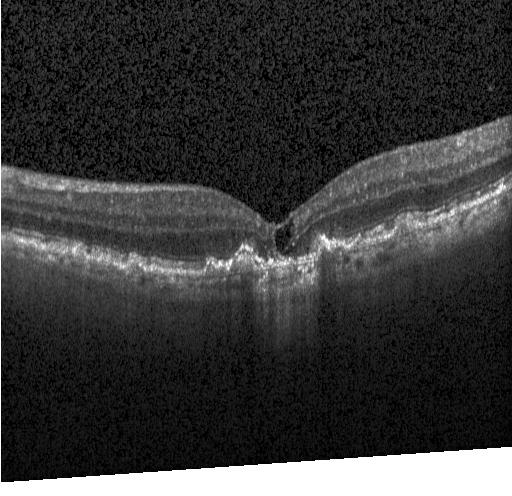

Heidelberg Spectralis OCT system, centered on the fovea, optical coherence tomography B-scan — Assessment: a choroidal neovascular membrane.